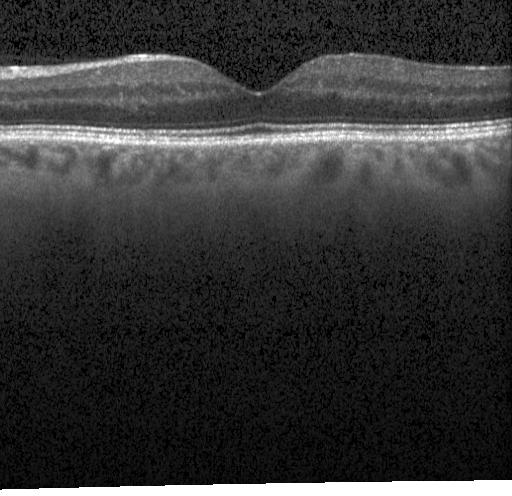
Impression: neither choroidal neovascularization, diabetic macular edema, nor drusen.